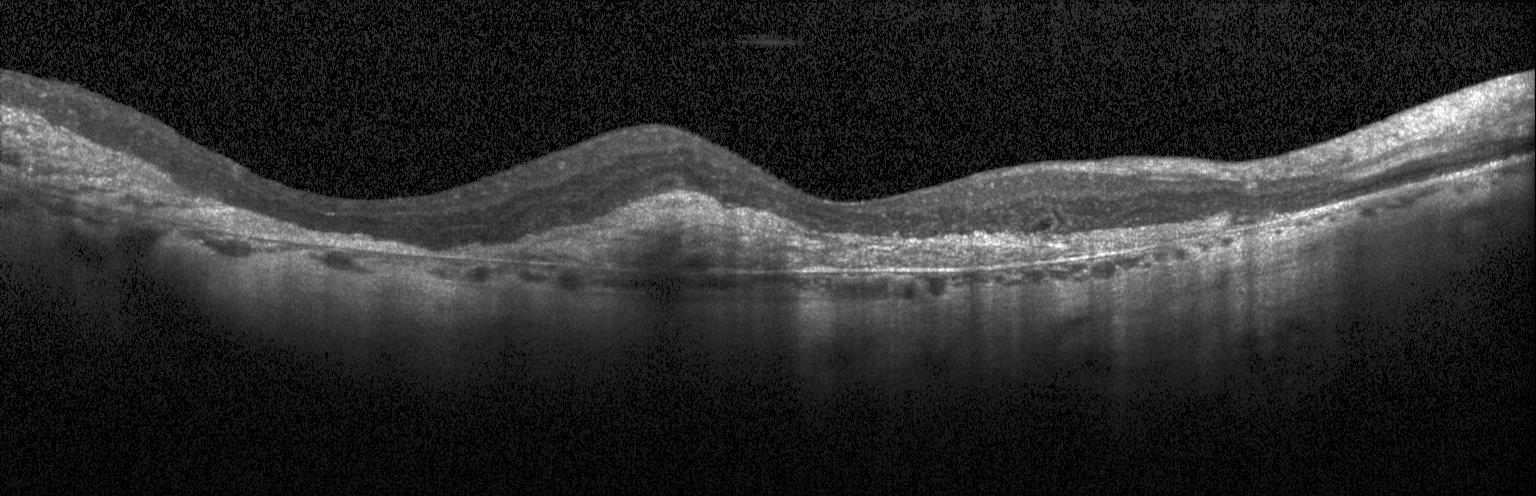 OCT line scan · SD-OCT — This B-scan demonstrates a choroidal neovascular membrane.